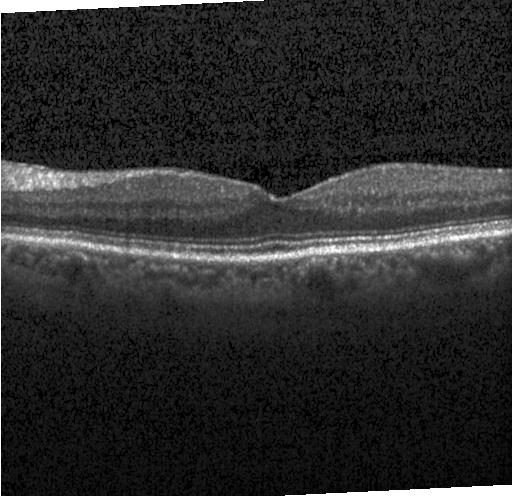

OCT line scan; Heidelberg Spectralis OCT system; centered on the fovea; spectral-domain optical coherence tomography — Finding: neither choroidal neovascularization, diabetic macular edema, nor drusen.